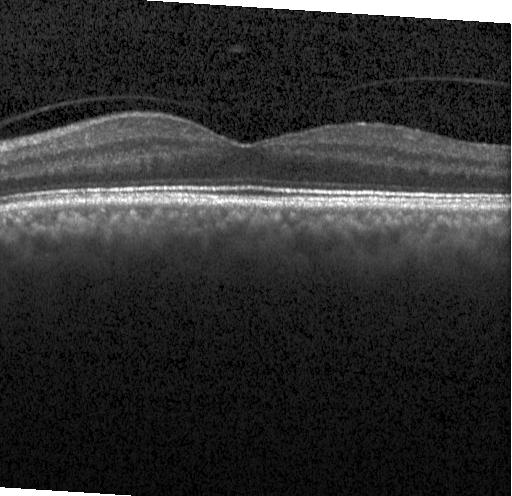
Macular OCT: no evidence of CNV, DME, or drusen.